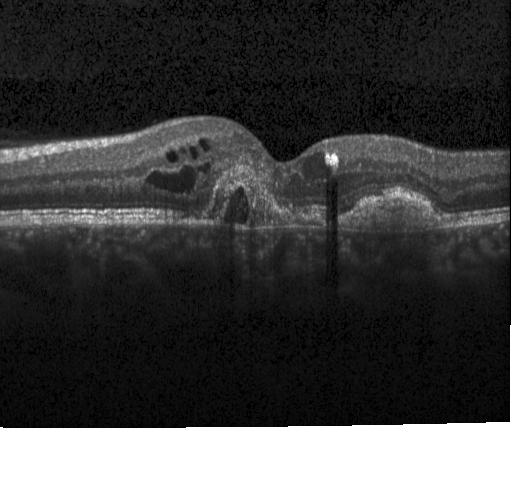 Impression: choroidal neovascularization (CNV).